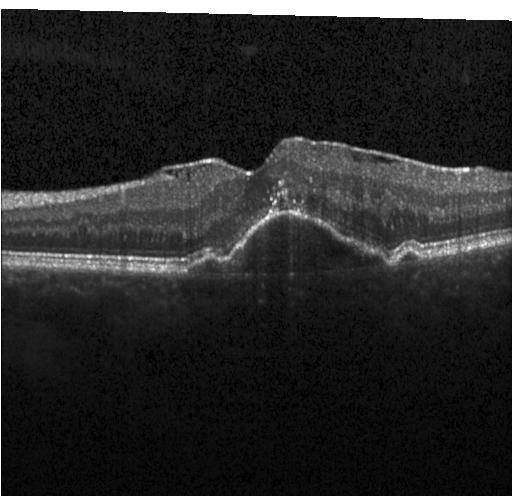

Through the macula, OCT B-scan. Dx: a choroidal neovascular membrane.